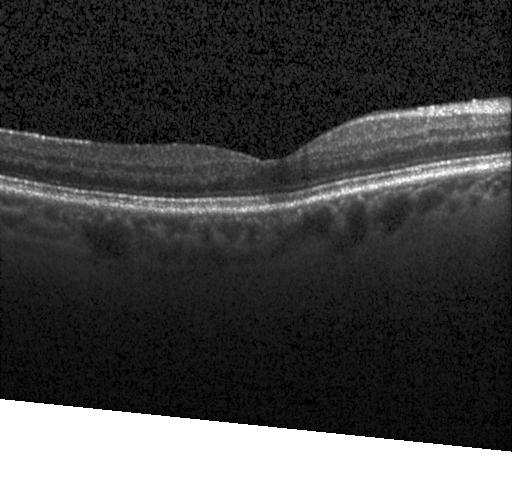 Retinal OCT cross-section, through the macula, spectral-domain OCT. The scan shows no evidence of choroidal neovascularization, diabetic macular edema, or drusen.